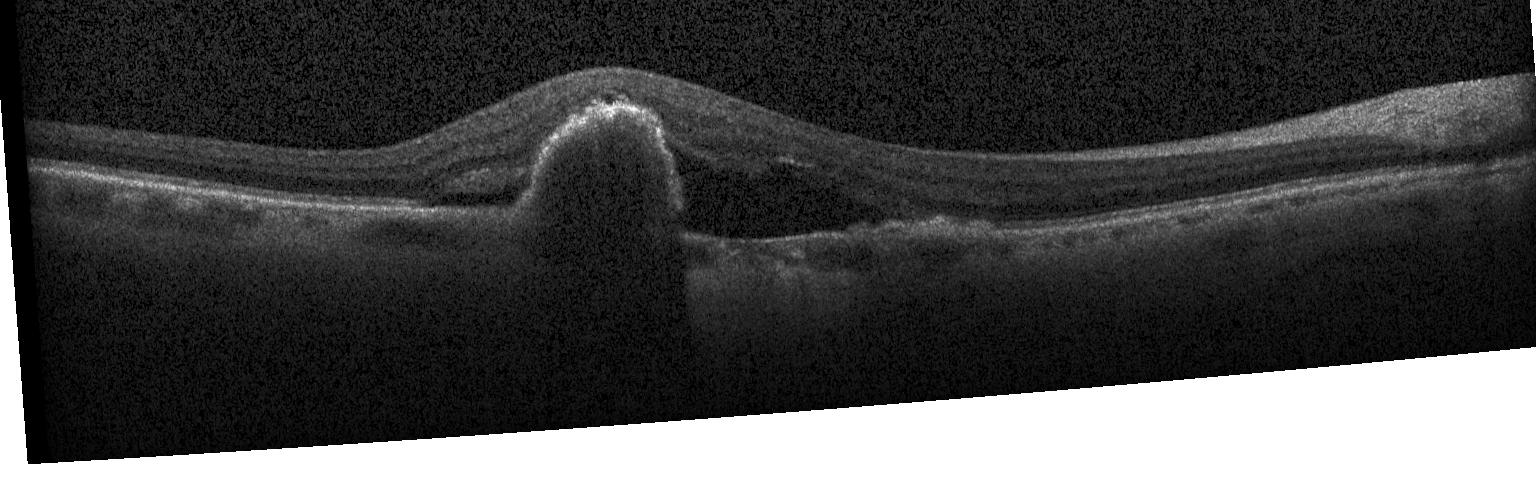
Dx: a choroidal neovascular membrane.